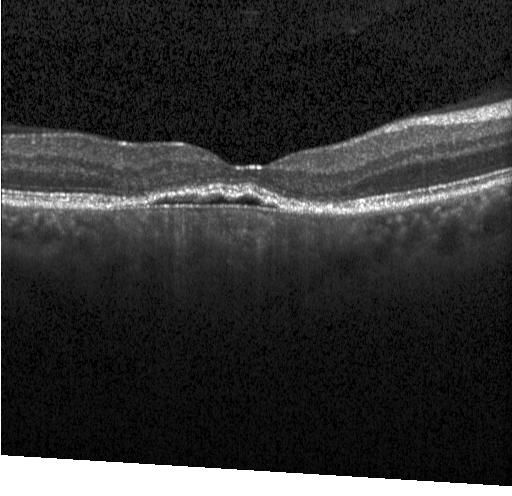

OCT line scan — Impression: CNV.